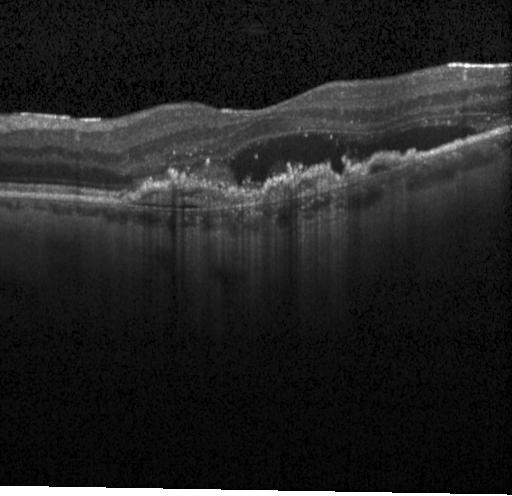
Acquired on a Heidelberg Spectralis; optical coherence tomography scan; horizontal scan through the fovea; SD-OCT.
Diagnosis: CNV.